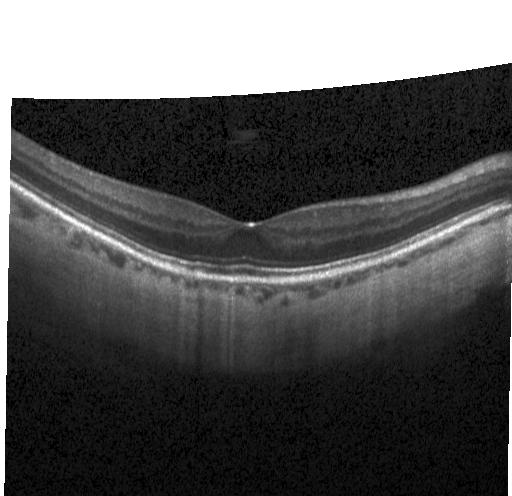

OCT line scan.
No evidence of CNV, DME, or drusen.